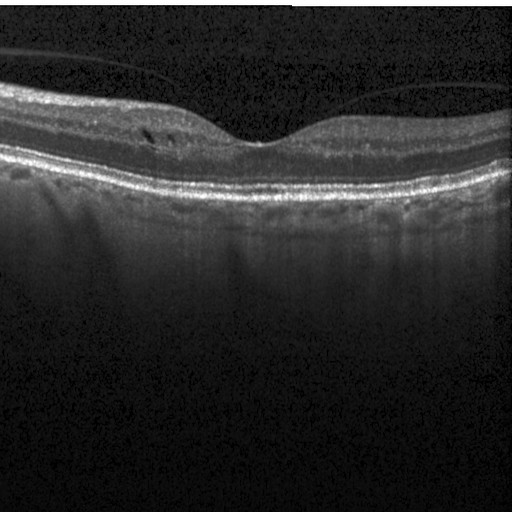 Acquired on a Heidelberg Spectralis. Optical coherence tomography B-scan. Diagnosis: diabetic macular edema.